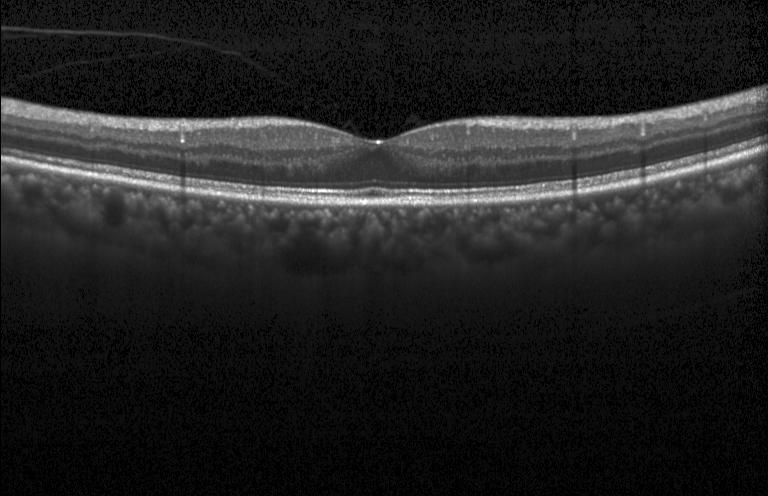

Retinal OCT cross-section — Assessment: no choroidal neovascularization, diabetic macular edema, or drusen.